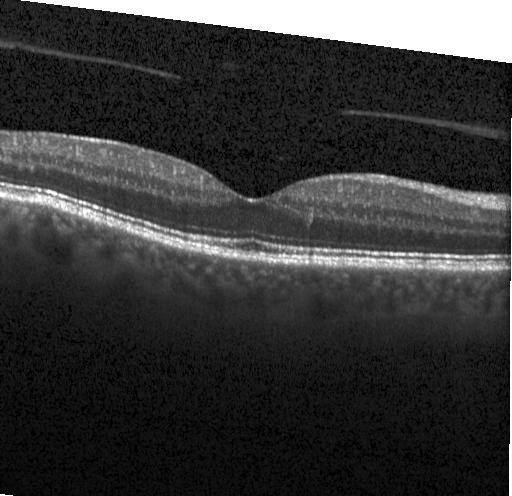
OCT B-scan showing no choroidal neovascularization, no diabetic macular edema, and no drusen.